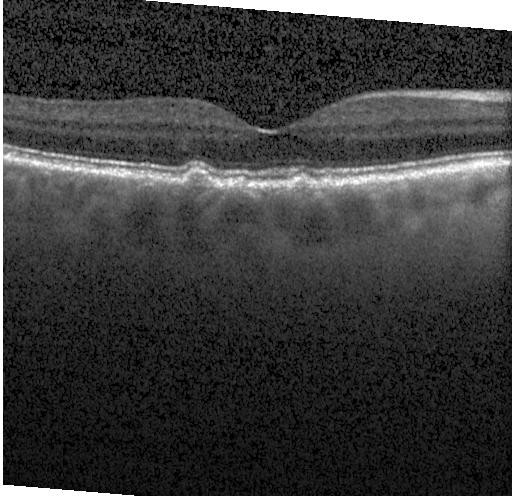
Retinal OCT cross-section; instrument: Heidelberg Spectralis. Finding: sub-RPE drusenoid deposits.